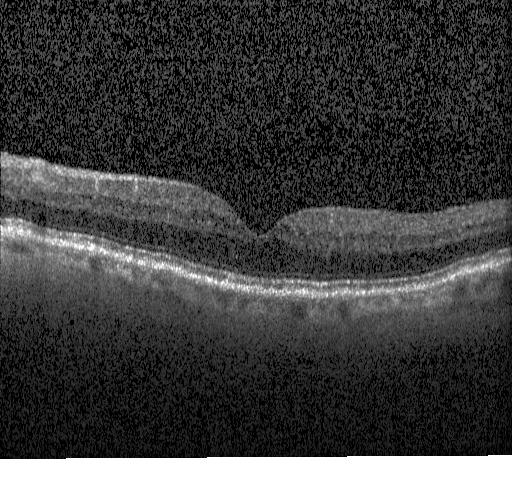
Spectral-domain OCT B-scan: no CNV, no DME, and no drusen.